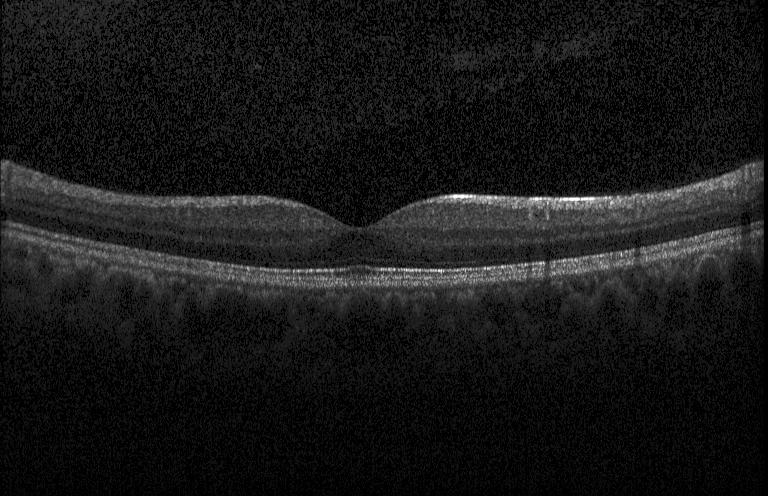 Fovea-centered; optical coherence tomography B-scan — Finding: no choroidal neovascularization, no diabetic macular edema, and no drusen.